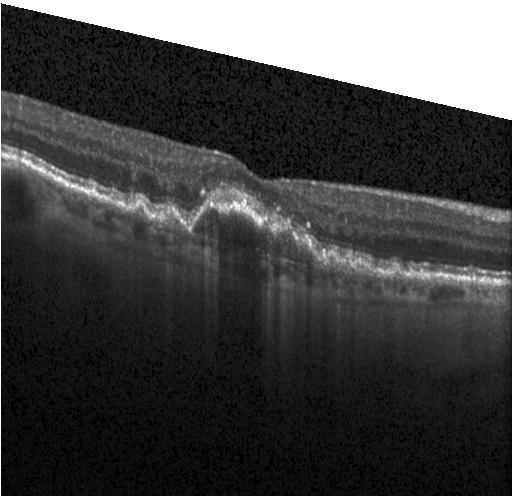
OCT line scan
Finding: a choroidal neovascular membrane.